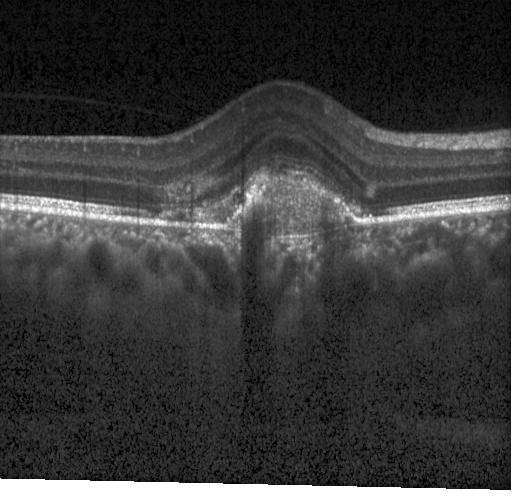
Macular OCT demonstrating a choroidal neovascular membrane.